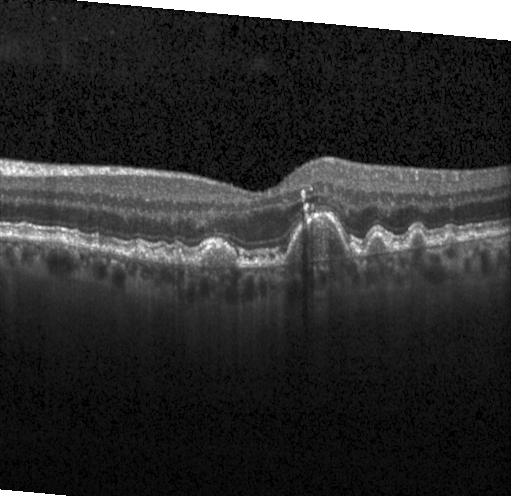 Instrument: Heidelberg Spectralis · macular scan · OCT line scan
The scan shows multiple drusen.